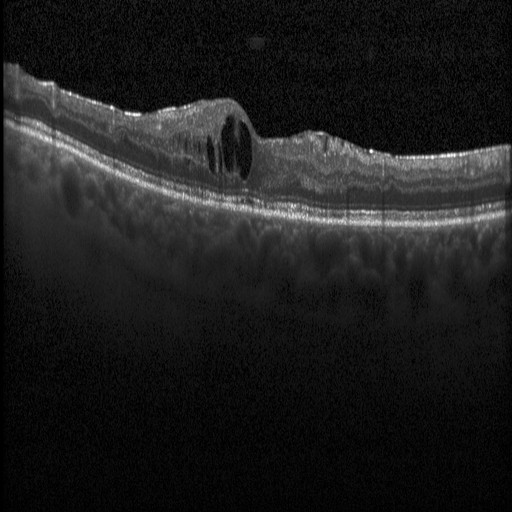 Horizontal scan through the fovea; optical coherence tomography B-scan.
Finding: DME.